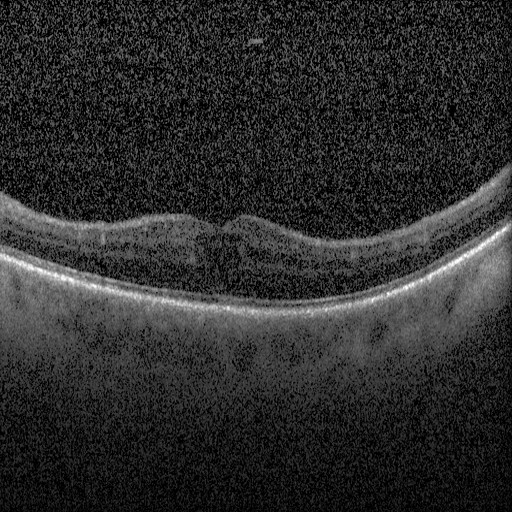
Dx: diabetic macular edema.